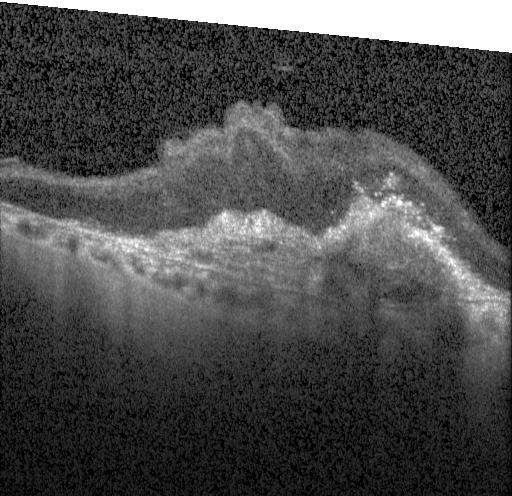
Choroidal neovascularization (CNV).